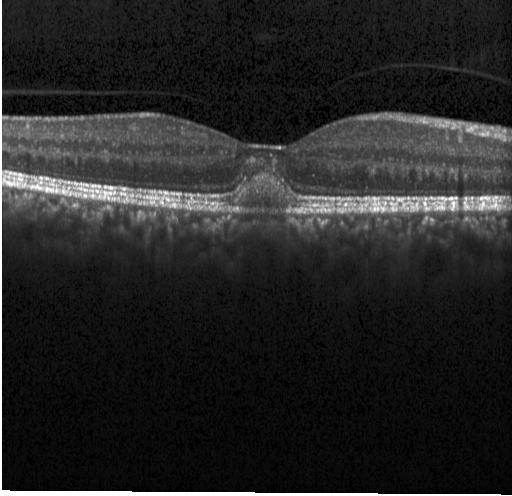

OCT B-scan
Impression: a choroidal neovascular membrane.